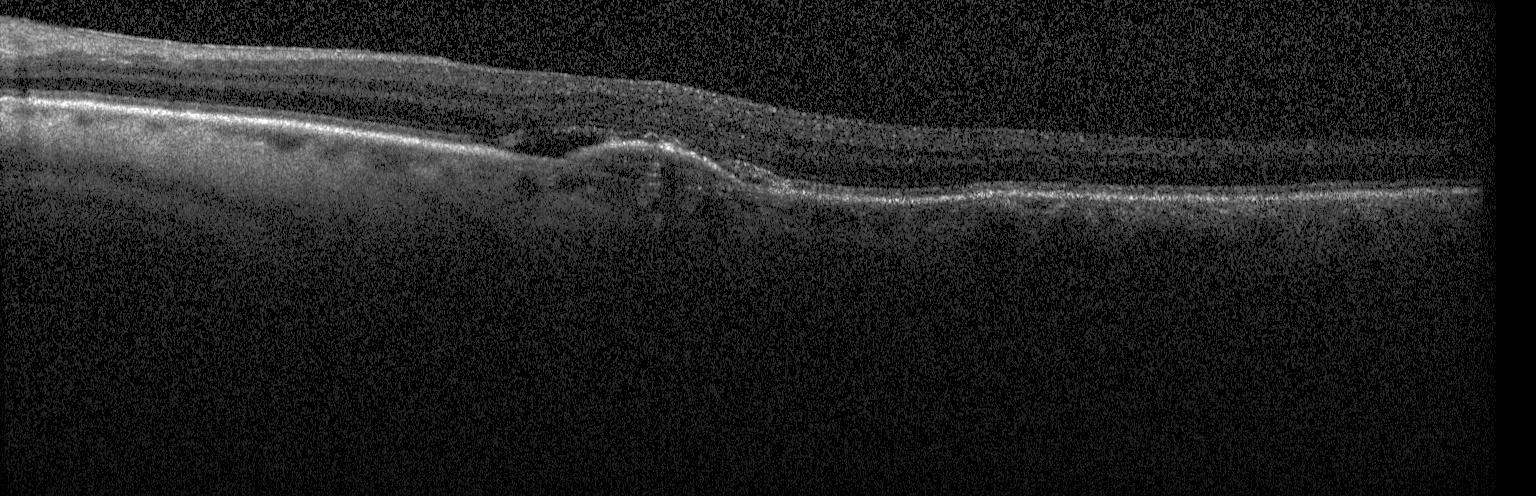 OCT B-scan; spectral-domain OCT — Finding: choroidal neovascularization (CNV).